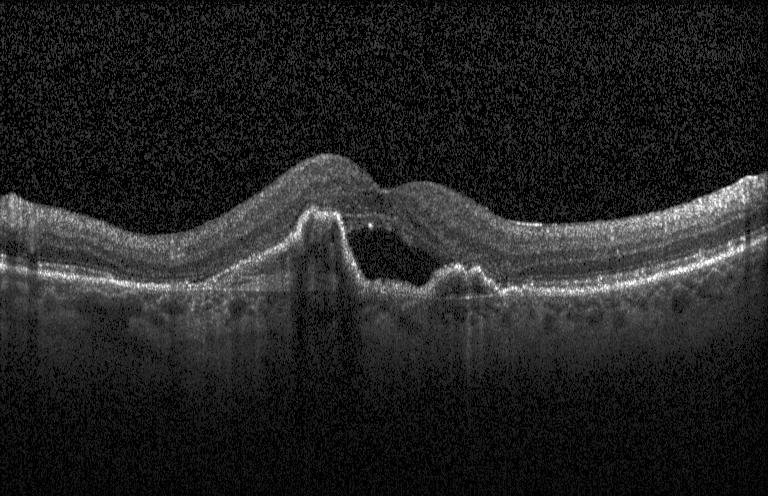

Diagnosis: CNV.